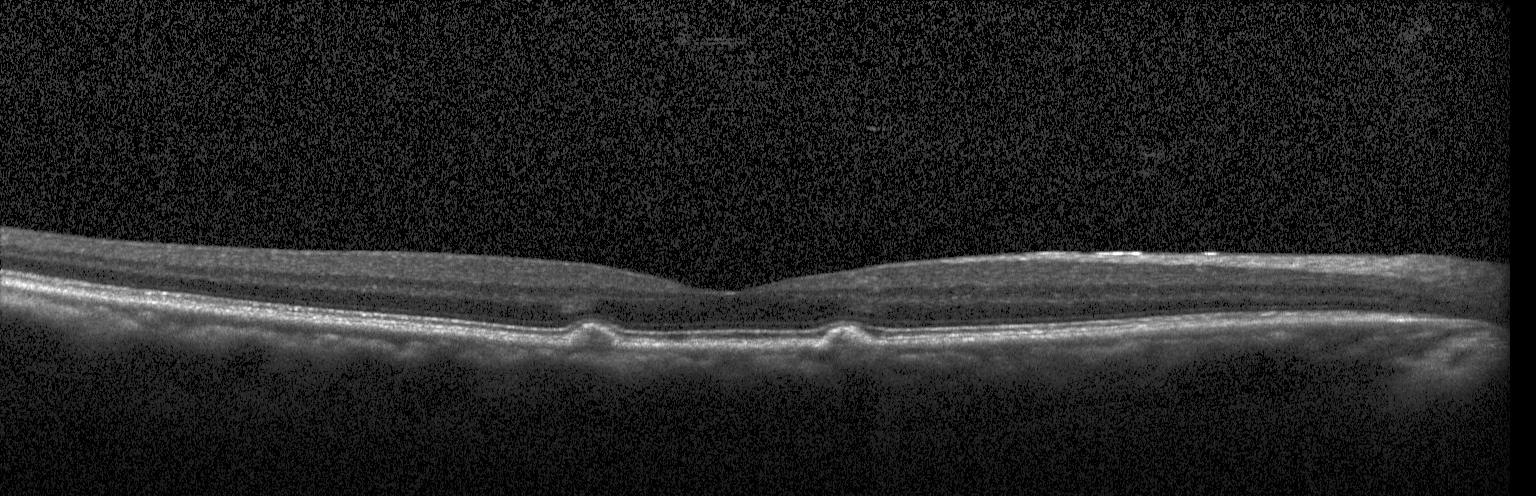 Multiple drusen.